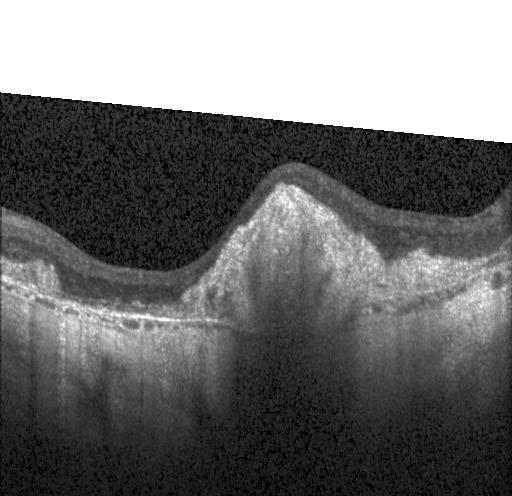
Optical coherence tomography scan.
Macular OCT: a choroidal neovascular membrane.